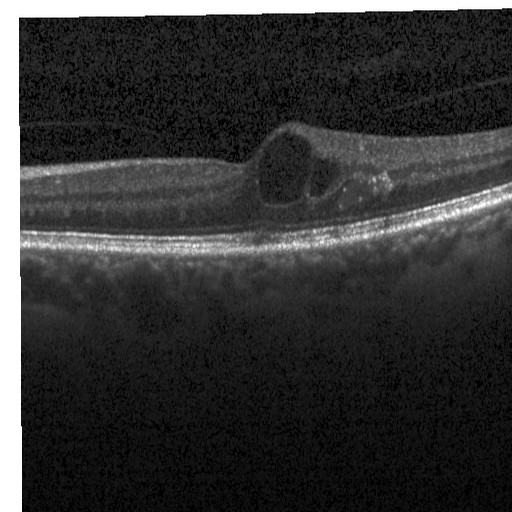 Dx: DME.